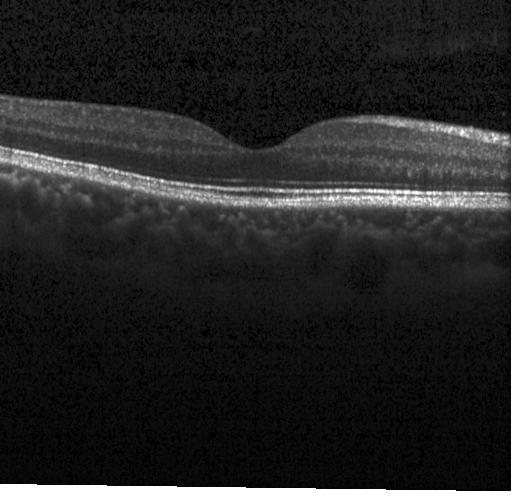

OCT scan showing no evidence of CNV, DME, or drusen.